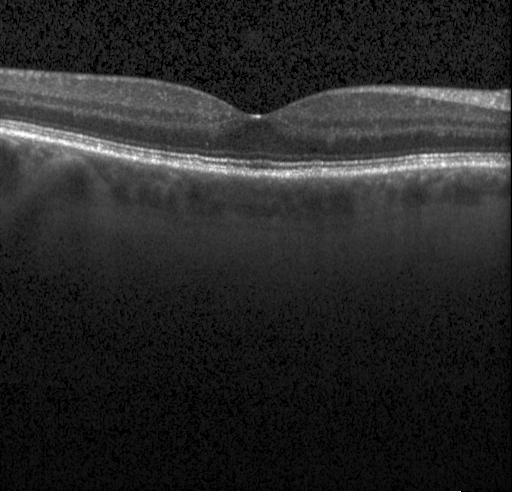 Horizontal scan through the fovea; SD-OCT; OCT line scan — Macular OCT: neither choroidal neovascularization, diabetic macular edema, nor drusen.